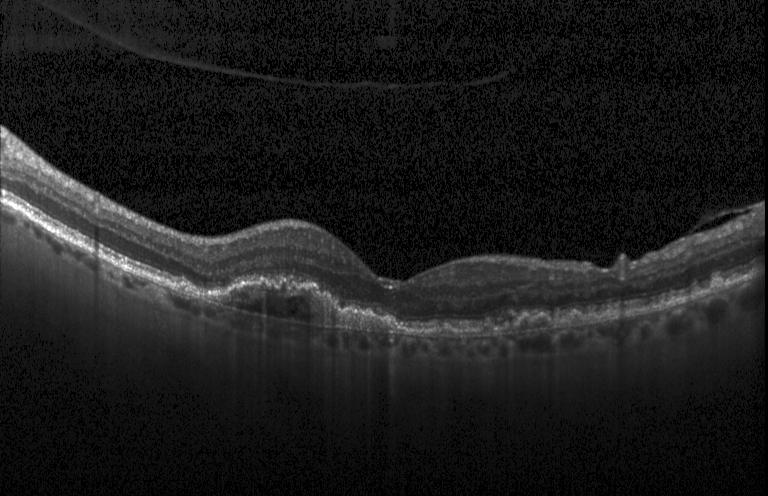
Acquired on a Heidelberg Spectralis. Spectral-domain optical coherence tomography. Retinal OCT B-scan — Diagnosis: choroidal neovascularization.